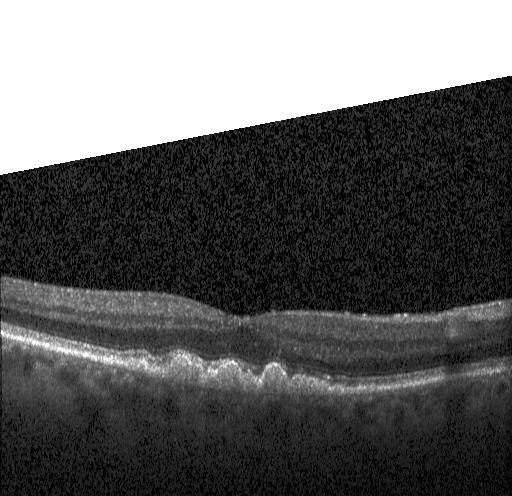
Spectral-domain OCT. Heidelberg Spectralis. OCT B-scan
The scan shows sub-RPE drusenoid deposits.